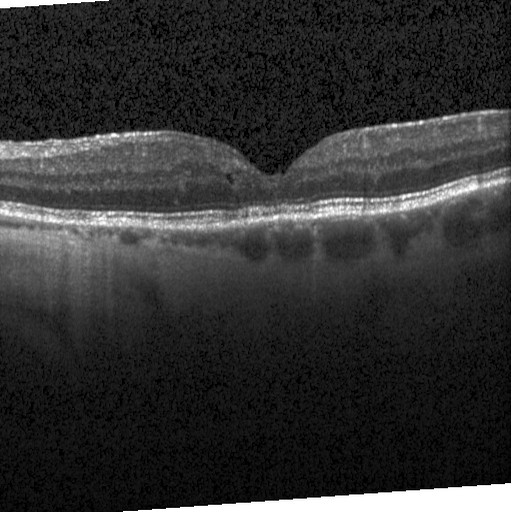 Retinal OCT cross-section; Heidelberg Spectralis OCT system; macular scan.
Finding: diabetic macular edema.